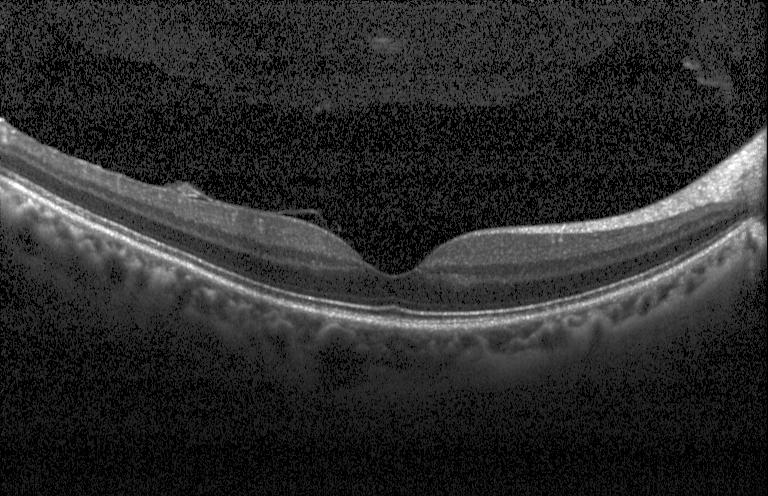

Acquired on a Heidelberg Spectralis, SD-OCT, OCT B-scan, through the macula. Assessment: no choroidal neovascularization, diabetic macular edema, or drusen.